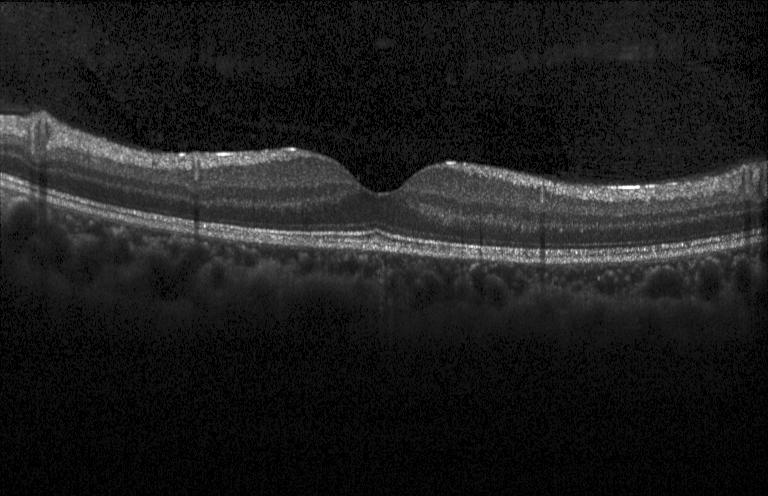 Spectral-domain OCT; optical coherence tomography B-scan; instrument: Heidelberg Spectralis; through the macula
Diagnosis: no CNV, DME, or drusen.